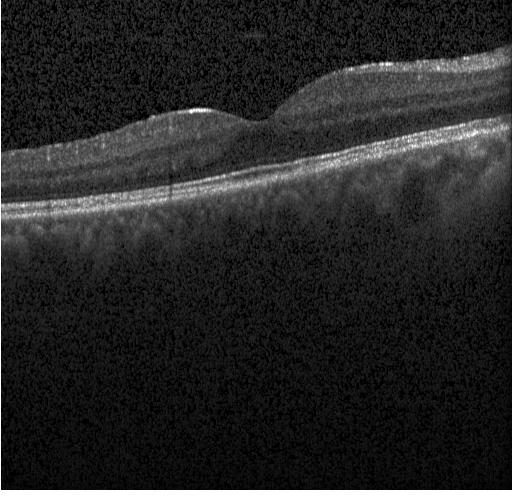 Centered on the fovea. Retinal OCT B-scan. Heidelberg Spectralis OCT system. Spectral-domain OCT — Finding: no CNV, DME, or drusen.